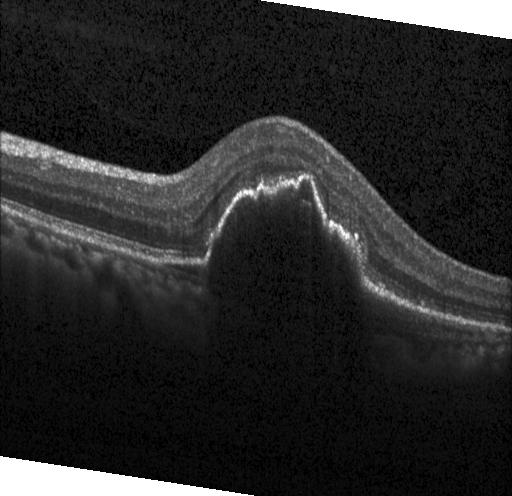 Optical coherence tomography B-scan. Diagnosis: a choroidal neovascular membrane.